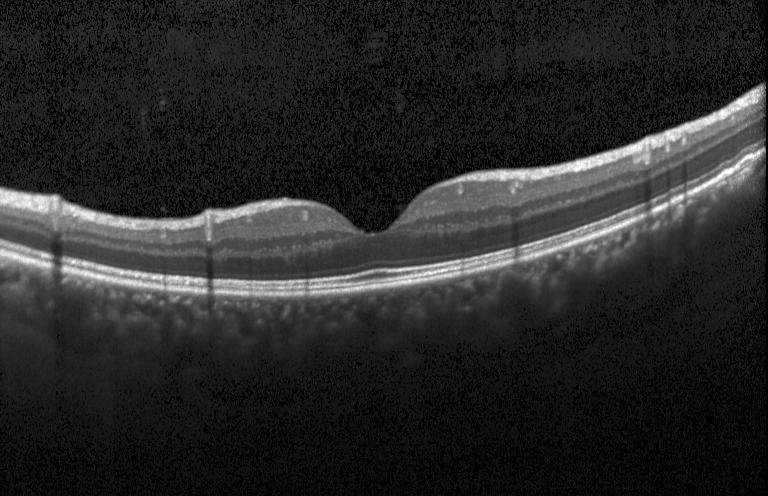
OCT scan showing no choroidal neovascularization, no diabetic macular edema, and no drusen.